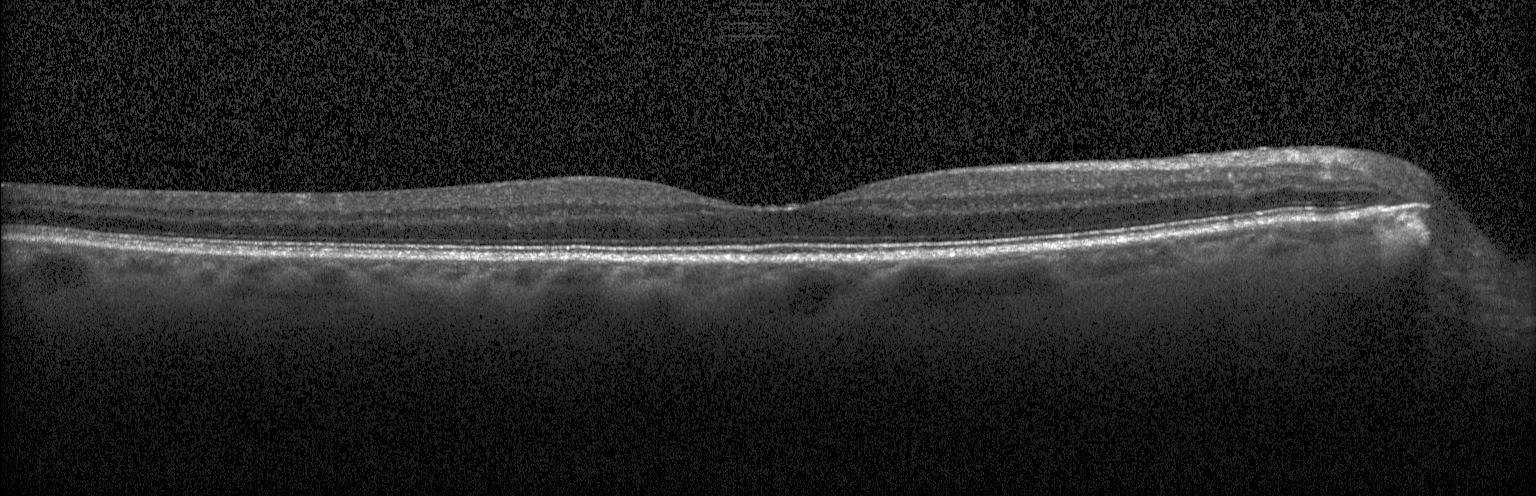

Spectral-domain OCT. Centered on the fovea. Acquired on a Heidelberg Spectralis. Retinal OCT B-scan — Diagnosis: no evidence of CNV, DME, or drusen.